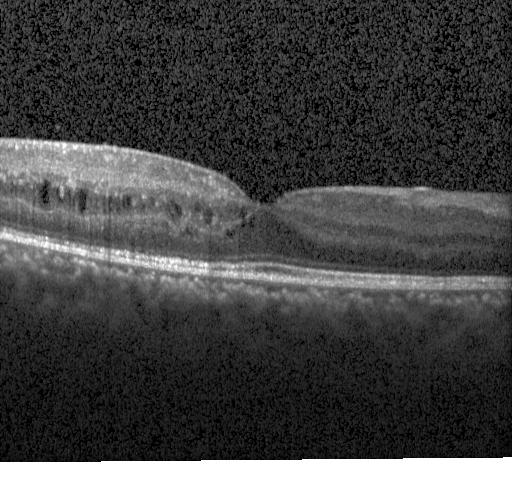 Macular scan; retinal OCT B-scan; SD-OCT.
Diagnosis: diabetic macular edema (DME).